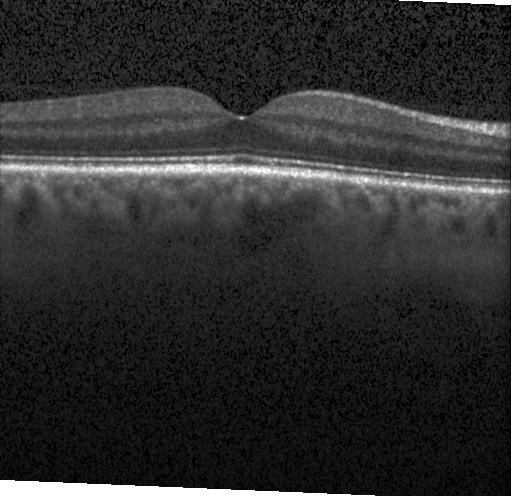 Finding: neither choroidal neovascularization, diabetic macular edema, nor drusen.